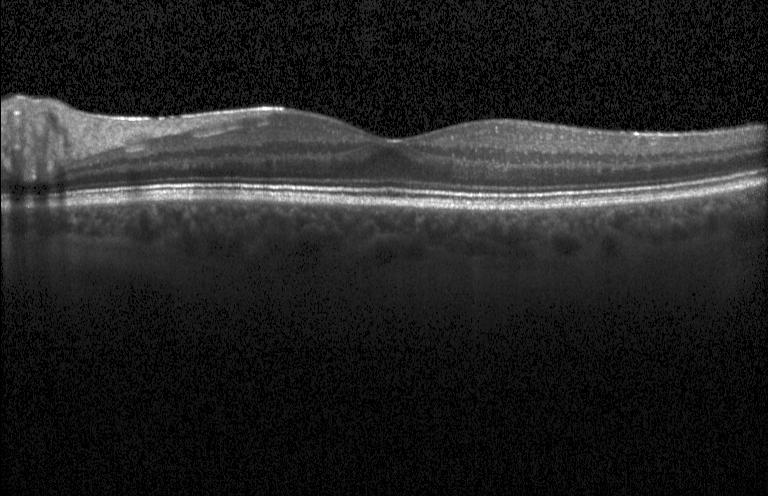

Diagnosis: neither CNV, DME, nor drusen.